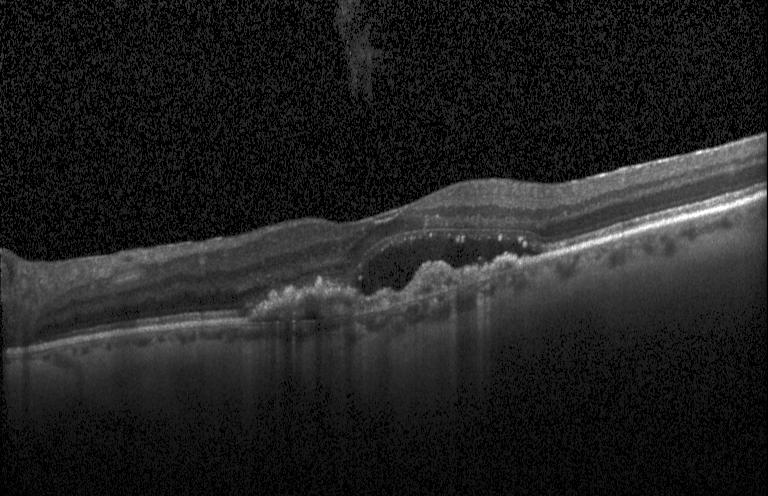

OCT finding: choroidal neovascularization (CNV).